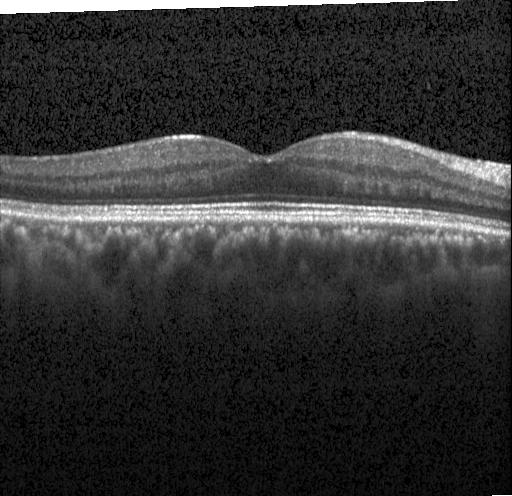 OCT line scan.
The scan shows no CNV, DME, or drusen.